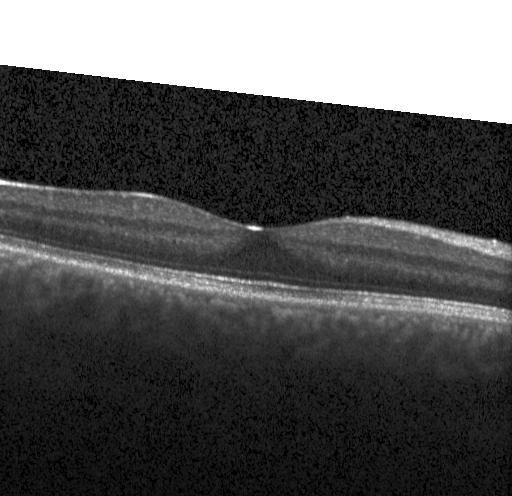

Heidelberg Spectralis OCT system, optical coherence tomography B-scan
The scan shows no choroidal neovascularization, no diabetic macular edema, and no drusen.